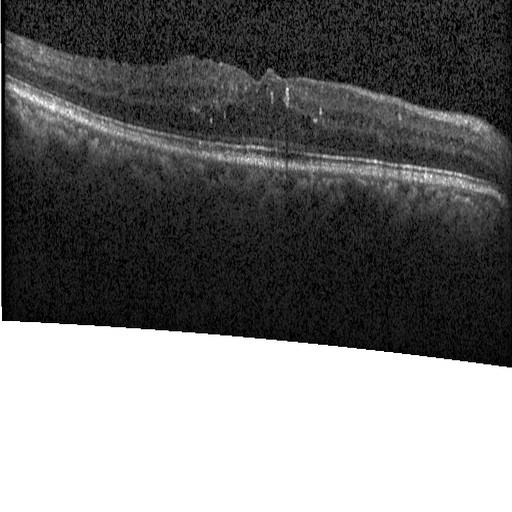 OCT scan showing diabetic macular edema.